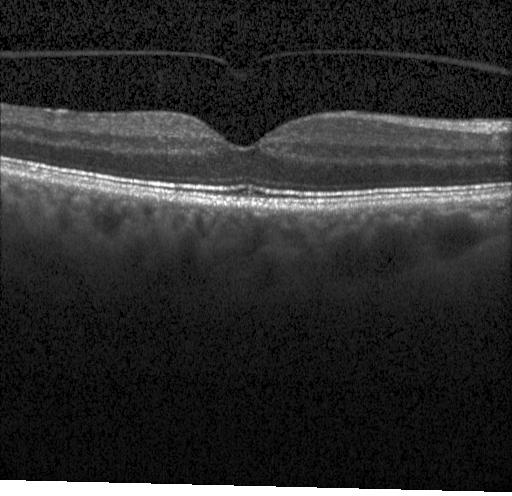
OCT scan showing neither choroidal neovascularization, diabetic macular edema, nor drusen.